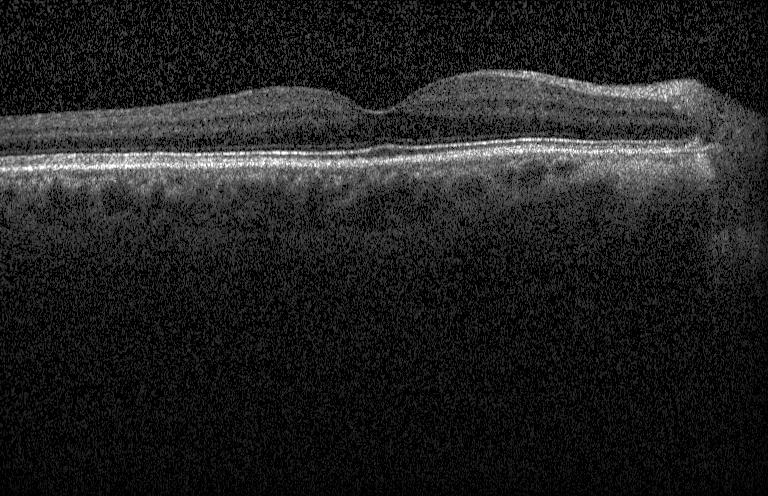
Retinal OCT B-scan; Heidelberg Spectralis OCT system; spectral-domain optical coherence tomography — Diagnosis: no evidence of choroidal neovascularization, diabetic macular edema, or drusen.